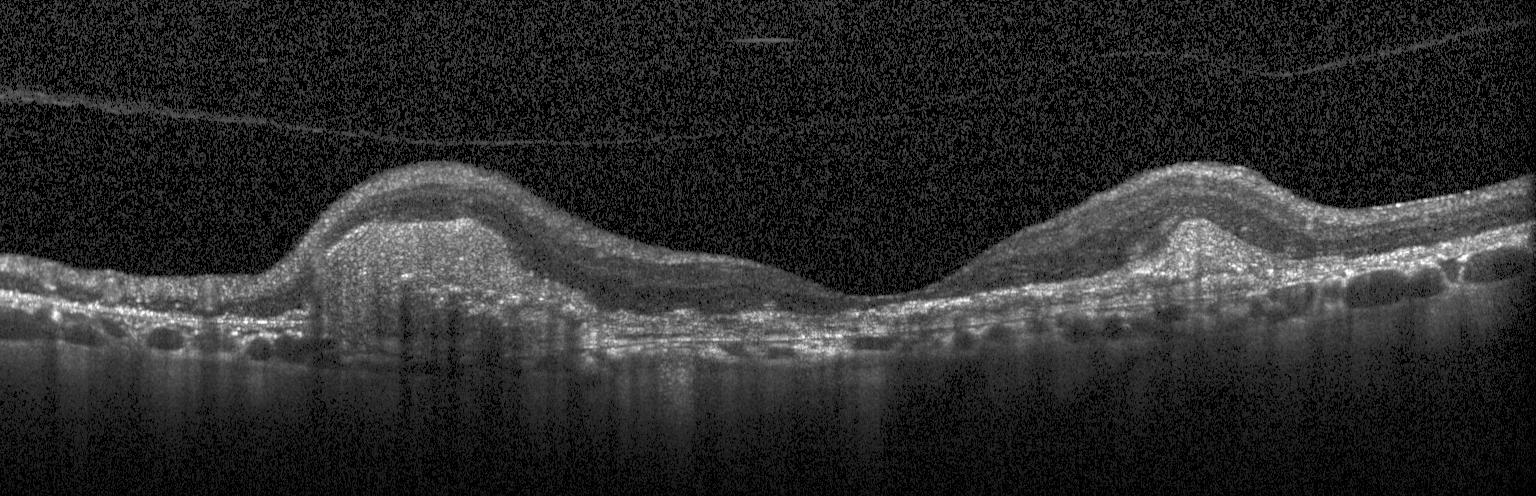 Spectral-domain OCT · macular scan · retinal OCT B-scan. Dx: a choroidal neovascular membrane.